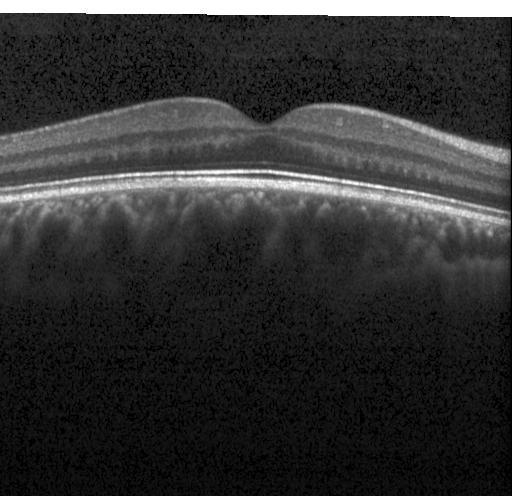
Optical coherence tomography scan · macular scan · spectral-domain OCT · acquired on a Heidelberg Spectralis. Dx: no choroidal neovascularization, diabetic macular edema, or drusen.